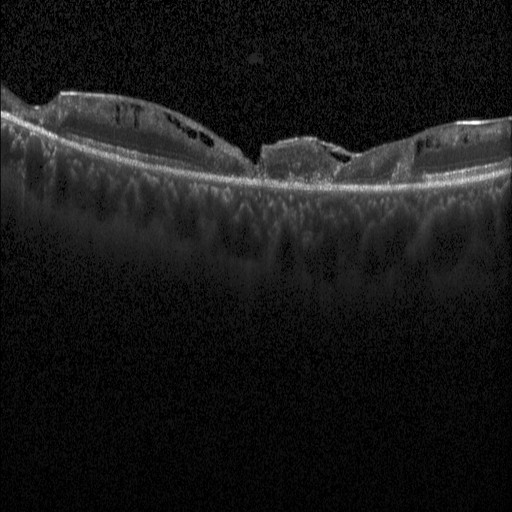

Heidelberg Spectralis OCT system. Spectral-domain optical coherence tomography. Horizontal scan through the fovea. OCT line scan
Diagnosis: diabetic macular edema (DME).